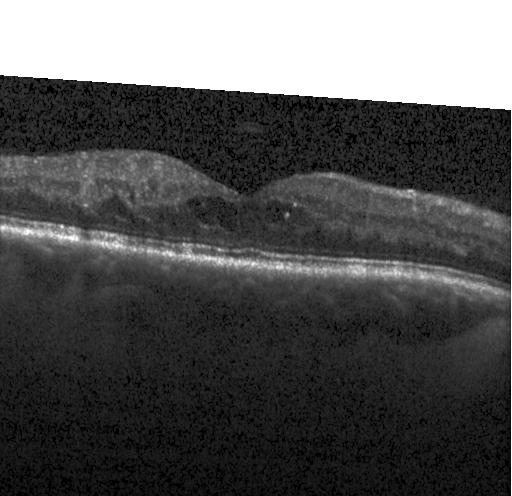
Retinal OCT B-scan
Impression: DME.